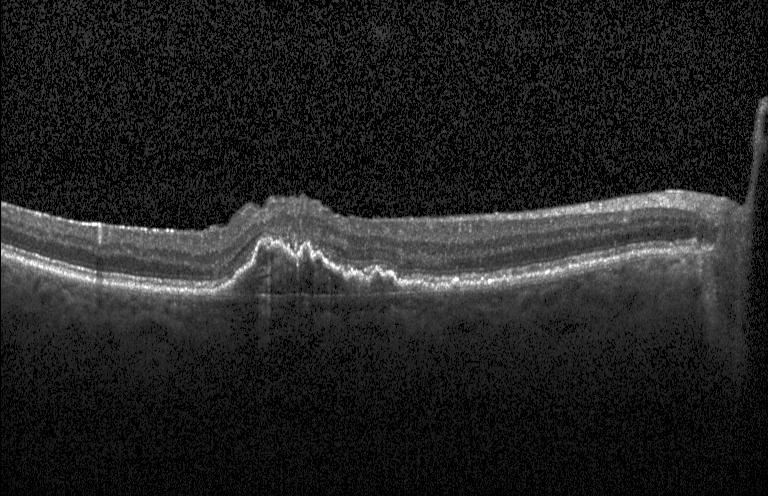

Retinal OCT cross-section. SD-OCT. Heidelberg Spectralis.
Impression: CNV.